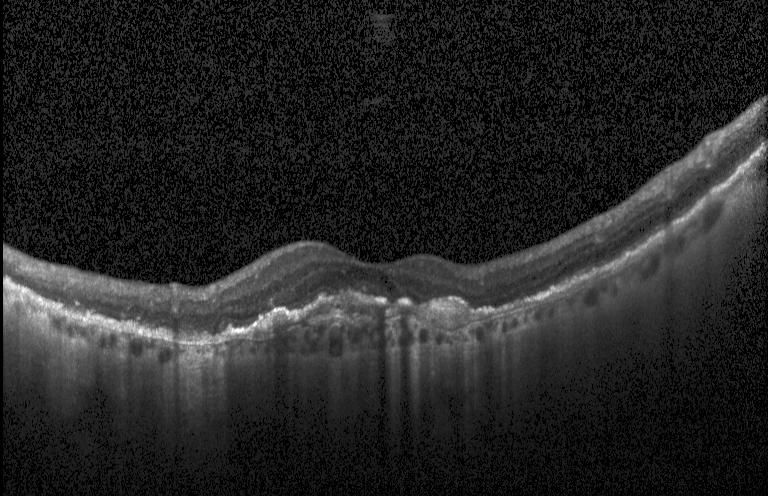

OCT B-scan. Heidelberg Spectralis OCT system
Diagnosis: a choroidal neovascular membrane.